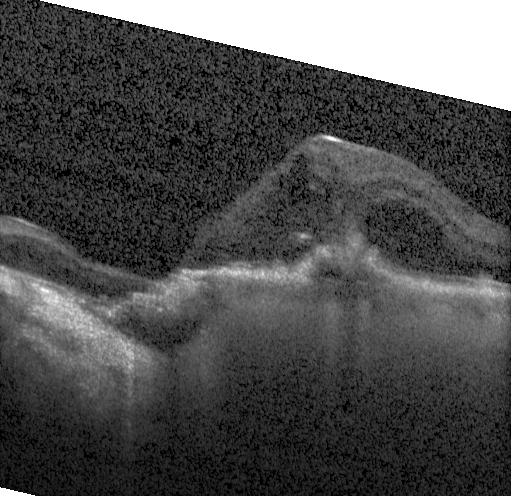 OCT line scan · Heidelberg Spectralis OCT system — This B-scan demonstrates a choroidal neovascular membrane.